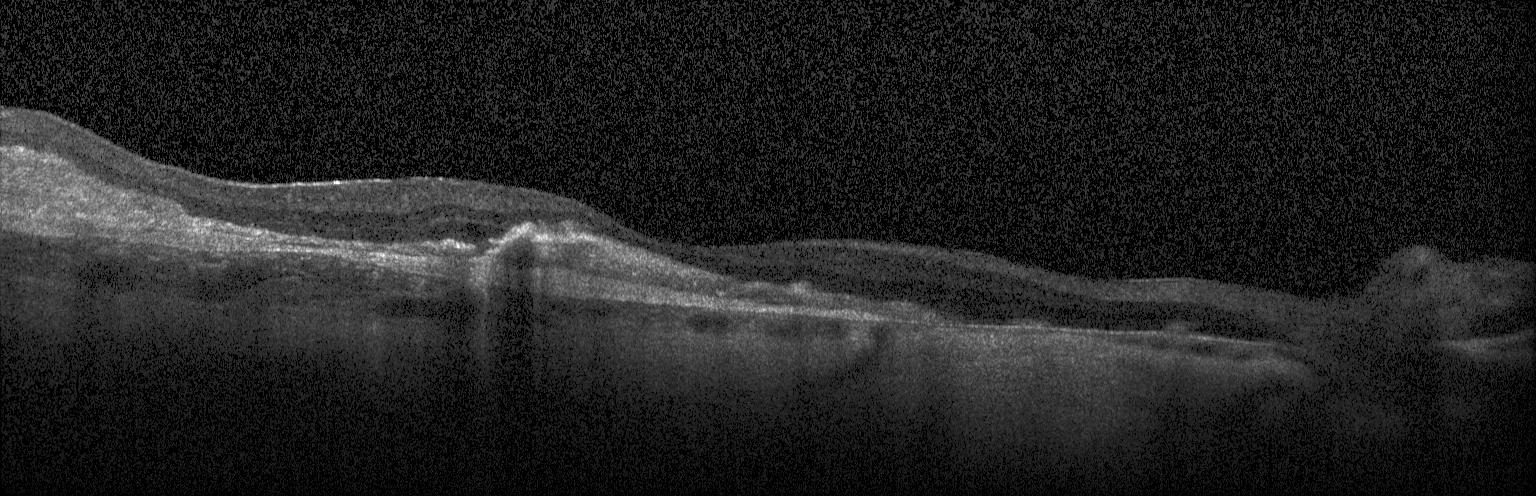 The scan shows choroidal neovascularization (CNV).